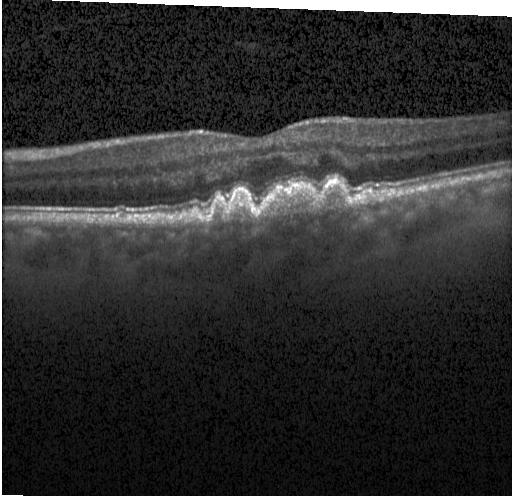
OCT B-scan; Heidelberg Spectralis
Assessment: a choroidal neovascular membrane.